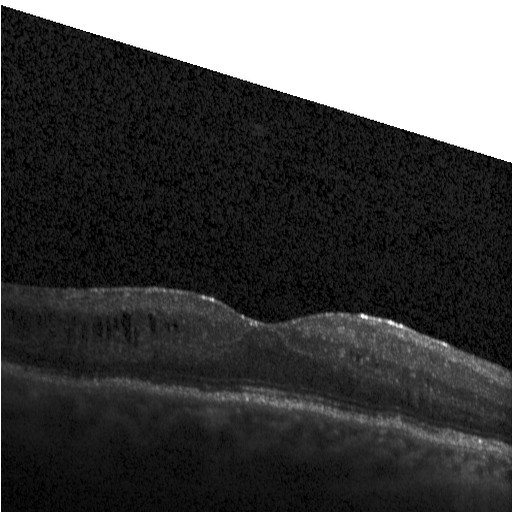
OCT B-scan — This B-scan demonstrates diabetic macular edema (DME).